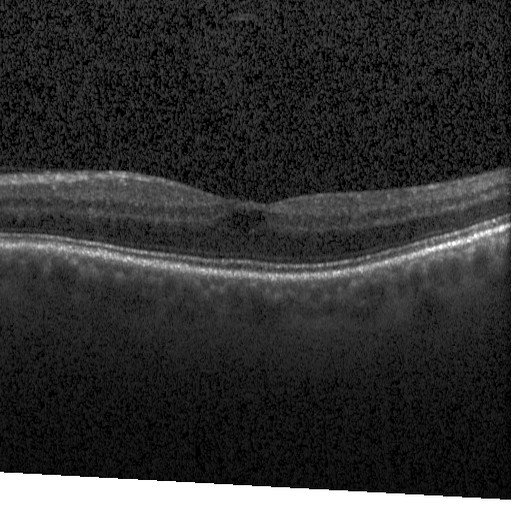

The scan shows DME.